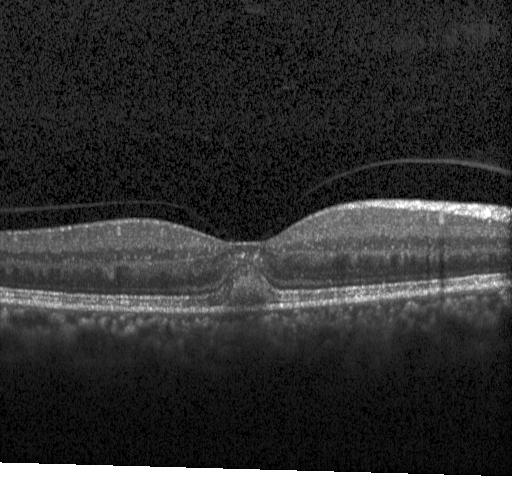

Dx: a choroidal neovascular membrane.